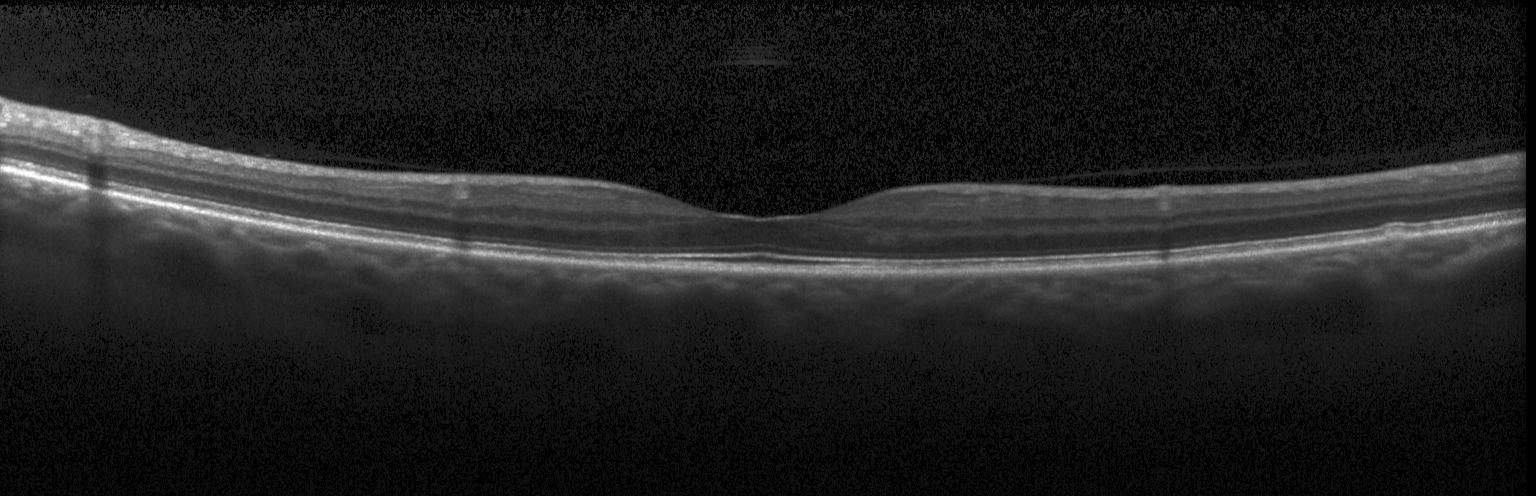
Spectral-domain optical coherence tomography · optical coherence tomography scan · Heidelberg Spectralis · centered on the fovea
Diagnosis: neither CNV, DME, nor drusen.